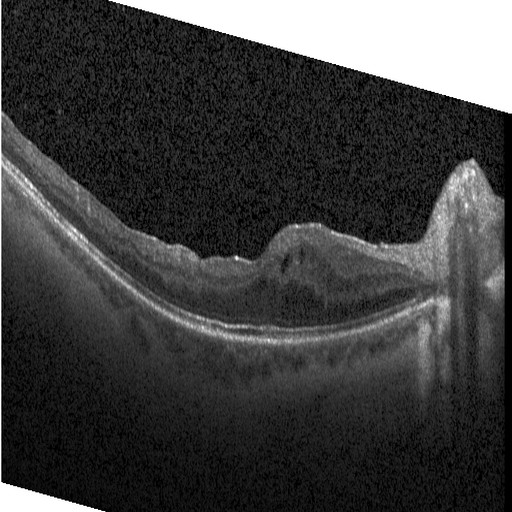 OCT B-scan showing diabetic macular edema.